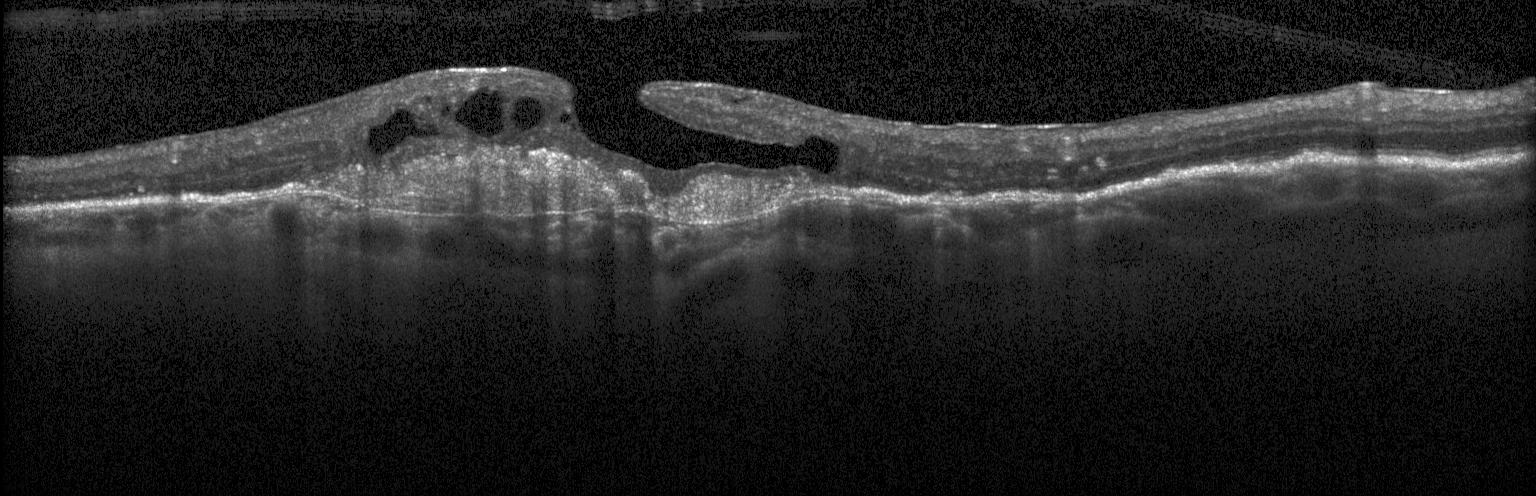 OCT B-scan showing choroidal neovascularization.